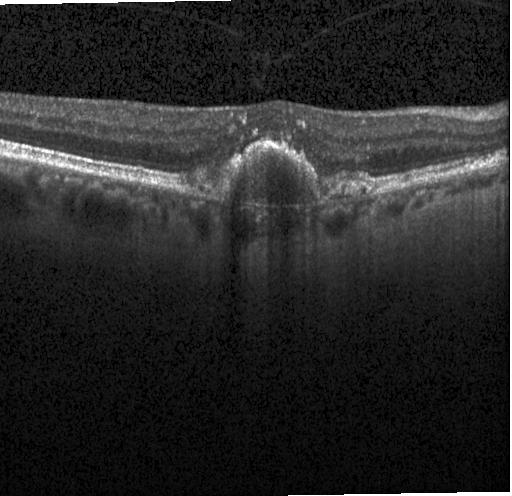
SD-OCT. Retinal OCT B-scan. Macular scan
Assessment: a choroidal neovascular membrane.